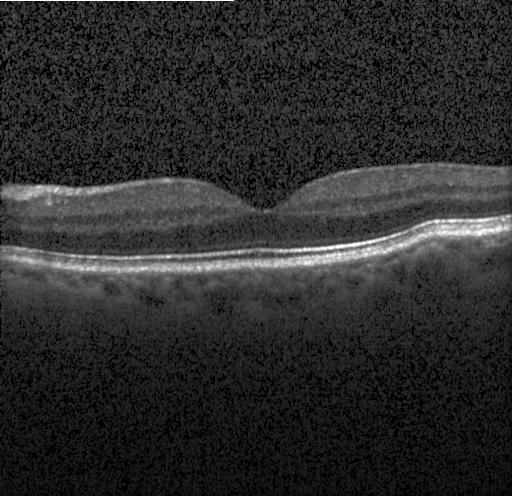
Finding: no choroidal neovascularization, no diabetic macular edema, and no drusen.